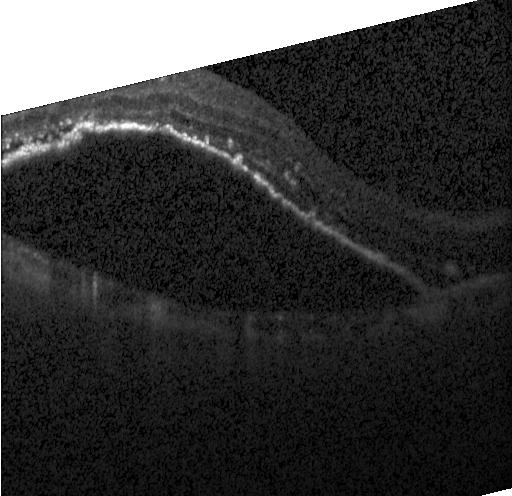 Retinal OCT B-scan.
Dx: a choroidal neovascular membrane.